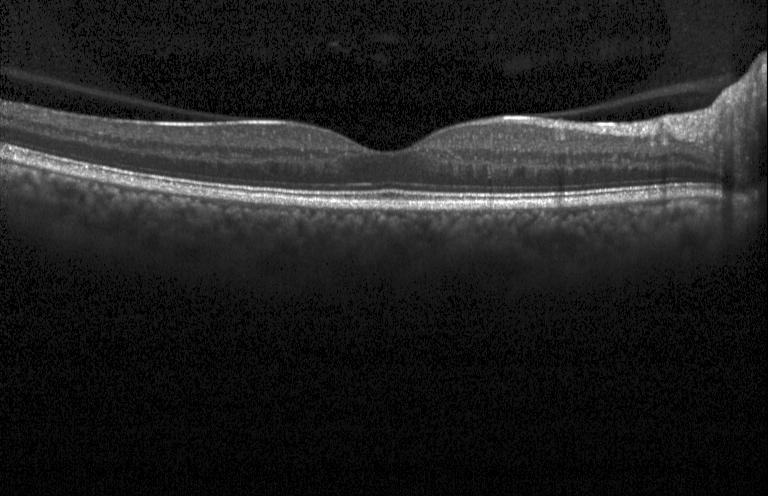

OCT B-scan showing neither choroidal neovascularization, diabetic macular edema, nor drusen.